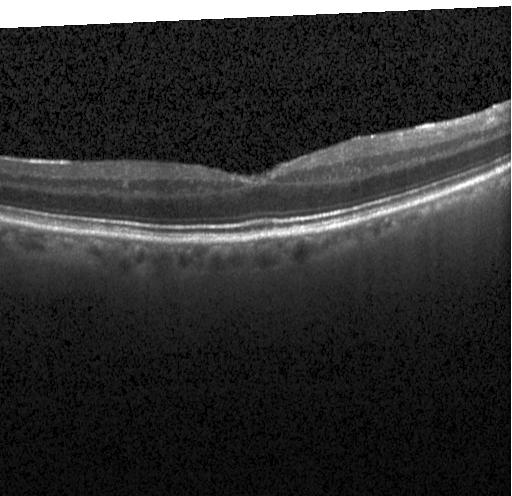

This B-scan demonstrates no CNV, no DME, and no drusen.